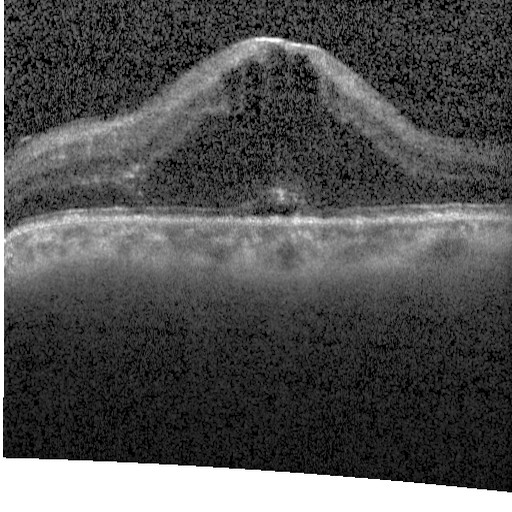

Optical coherence tomography B-scan — Diabetic macular edema.